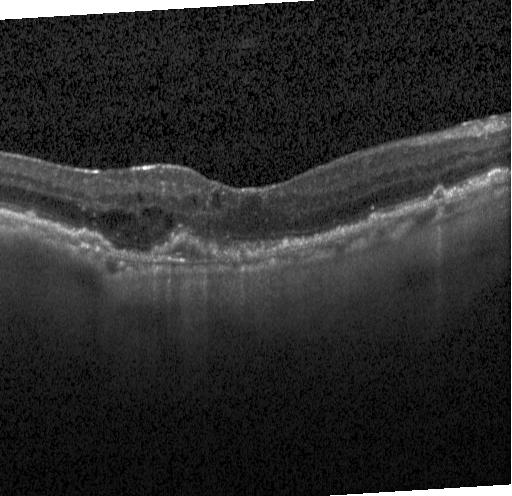

The scan shows a choroidal neovascular membrane.